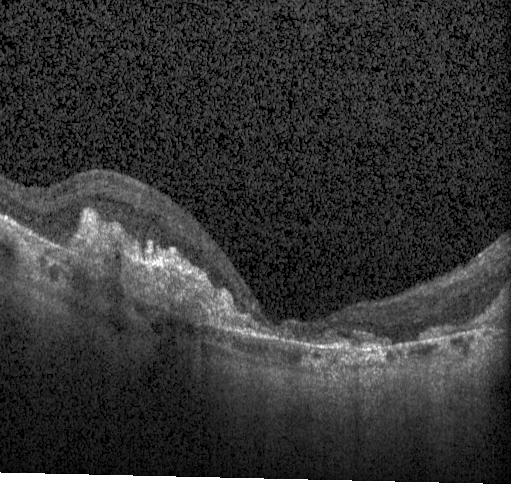
Dx: a choroidal neovascular membrane.